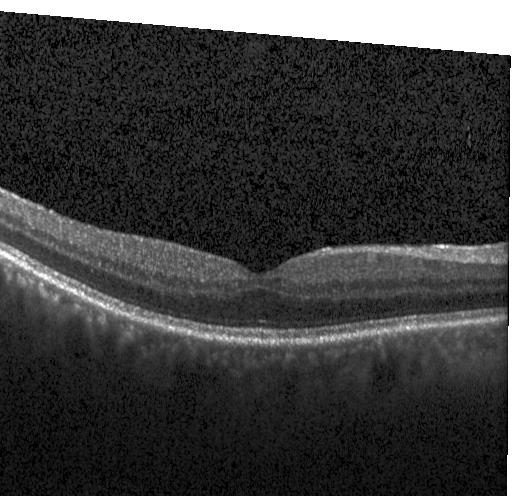

Retinal OCT B-scan. Dx: no choroidal neovascularization, no diabetic macular edema, and no drusen.